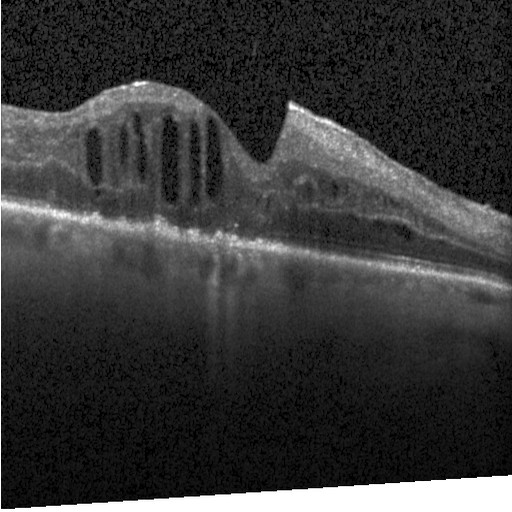
OCT line scan. Dx: DME.